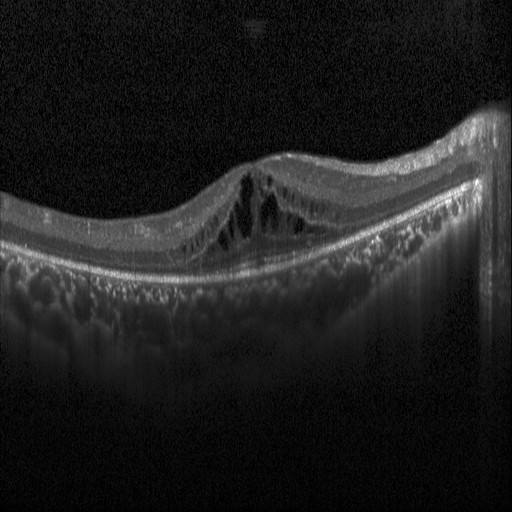 OCT B-scan · spectral-domain optical coherence tomography.
Diagnosis: DME.